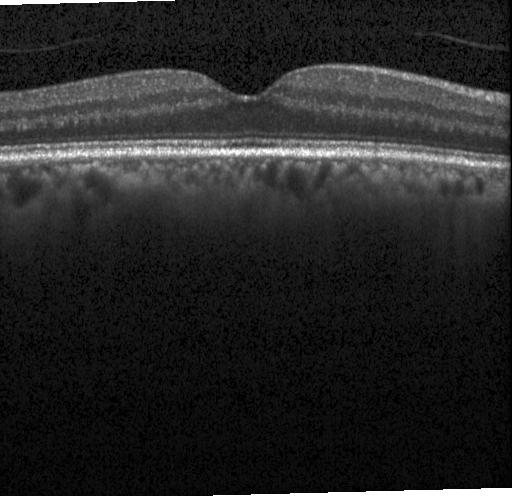 Optical coherence tomography B-scan.
Impression: no evidence of CNV, DME, or drusen.